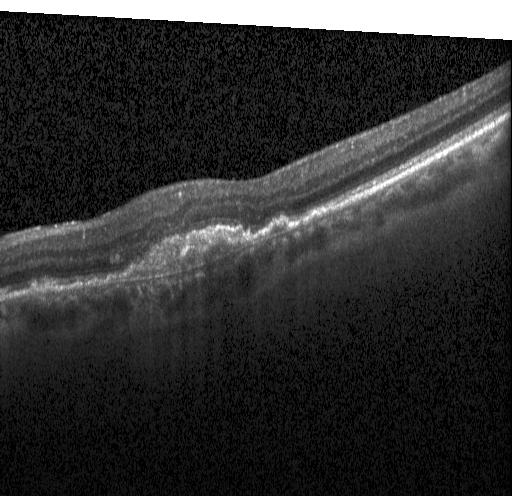 Optical coherence tomography B-scan · macular scan — The scan shows choroidal neovascularization.